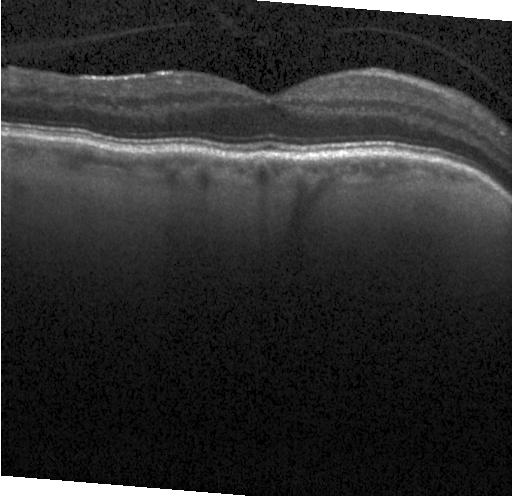 Neither choroidal neovascularization, diabetic macular edema, nor drusen.